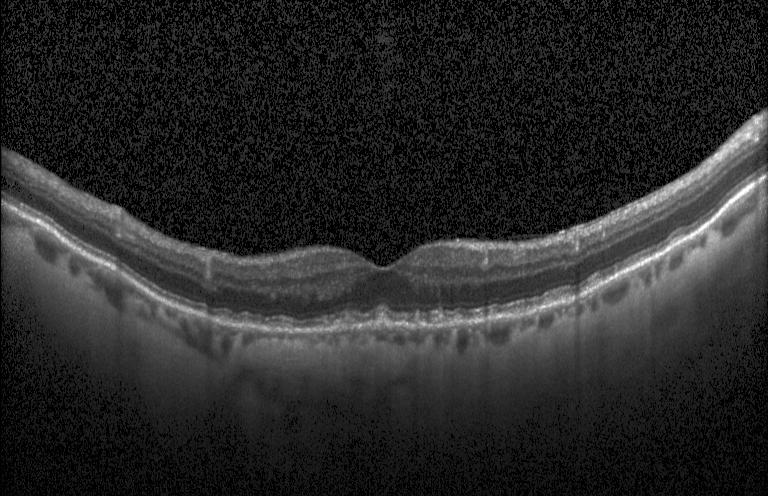
Retinal OCT cross-section showing multiple drusen.